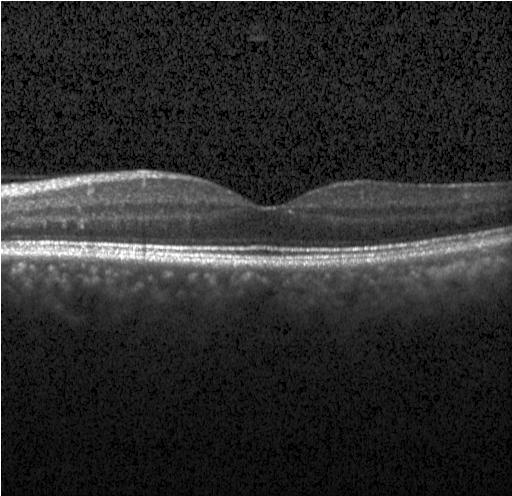

Retinal OCT B-scan.
This B-scan demonstrates no choroidal neovascularization, no diabetic macular edema, and no drusen.